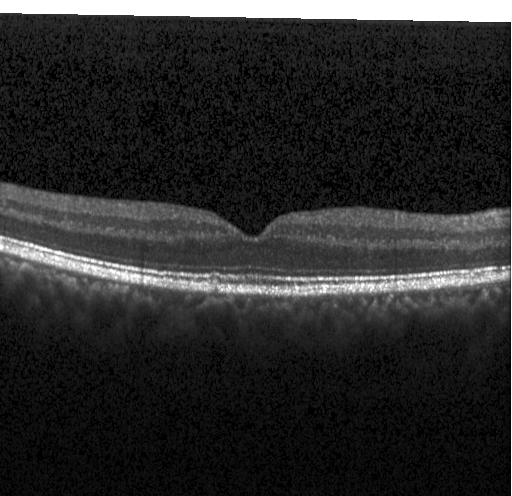

Heidelberg Spectralis, retinal OCT cross-section
The scan shows neither CNV, DME, nor drusen.